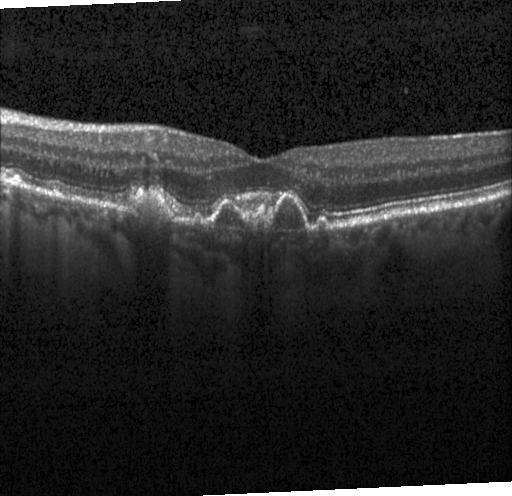

OCT B-scan · acquired on a Heidelberg Spectralis — Choroidal neovascularization.